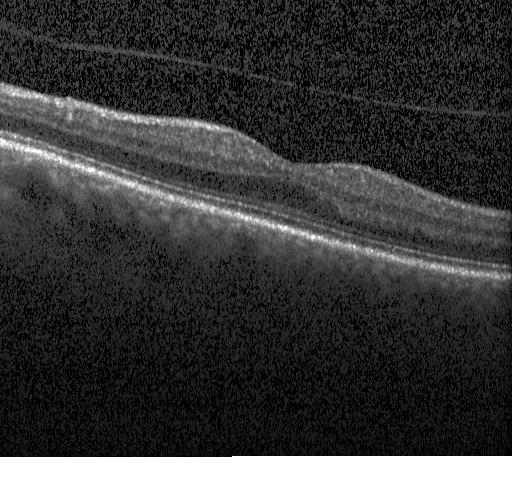
Heidelberg Spectralis, retinal OCT B-scan — Diagnosis: no evidence of choroidal neovascularization, diabetic macular edema, or drusen.